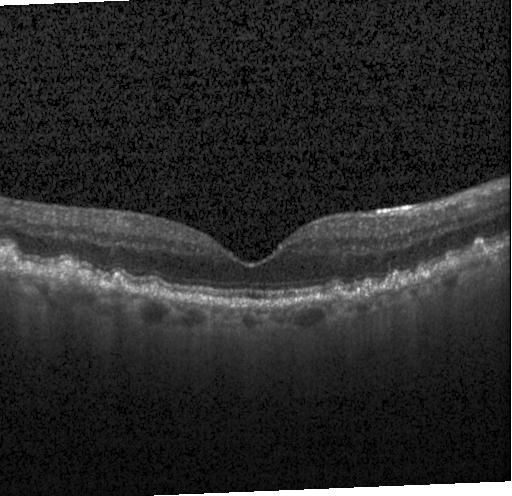

OCT line scan. Spectral-domain optical coherence tomography. Impression: multiple drusen.